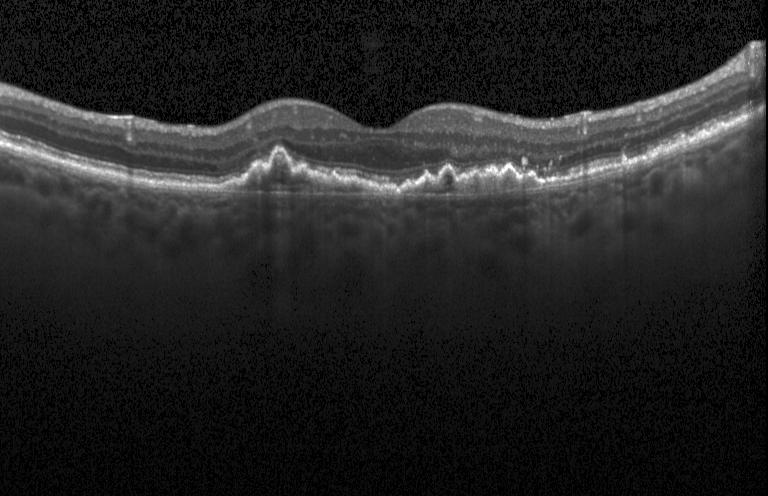
Optical coherence tomography scan, fovea-centered — Impression: choroidal neovascularization.